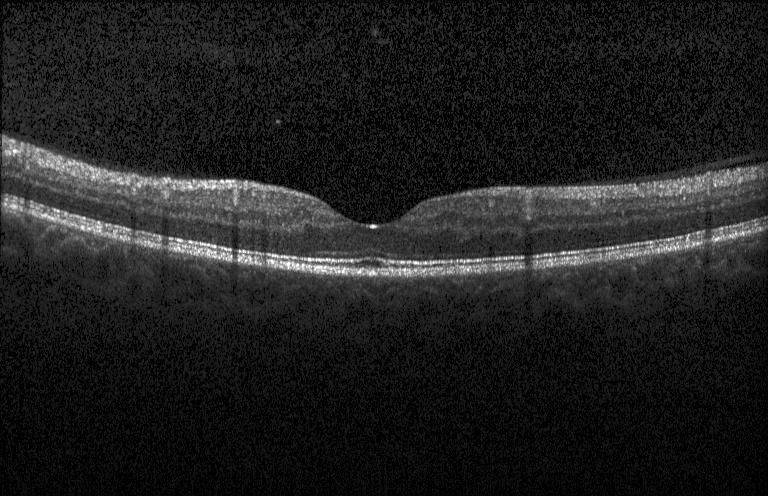
Impression: no choroidal neovascularization, diabetic macular edema, or drusen.